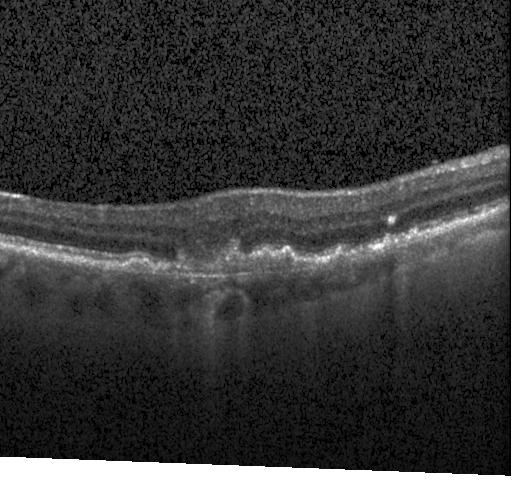
SD-OCT · retinal OCT B-scan — CNV.